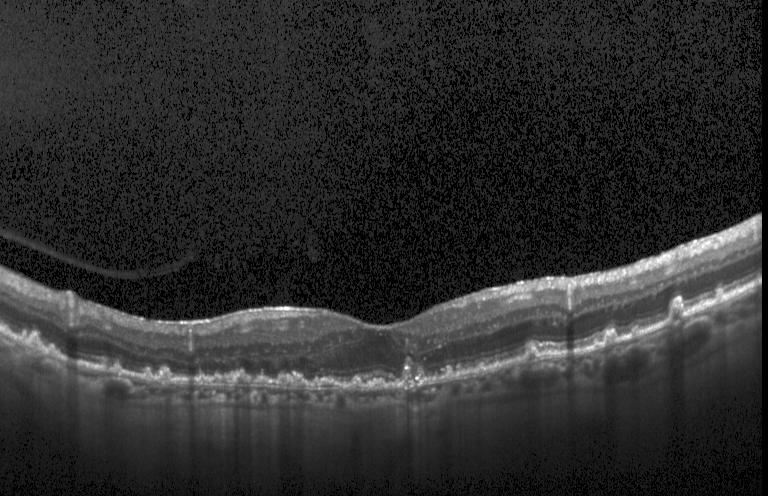
Diagnosis: a choroidal neovascular membrane.